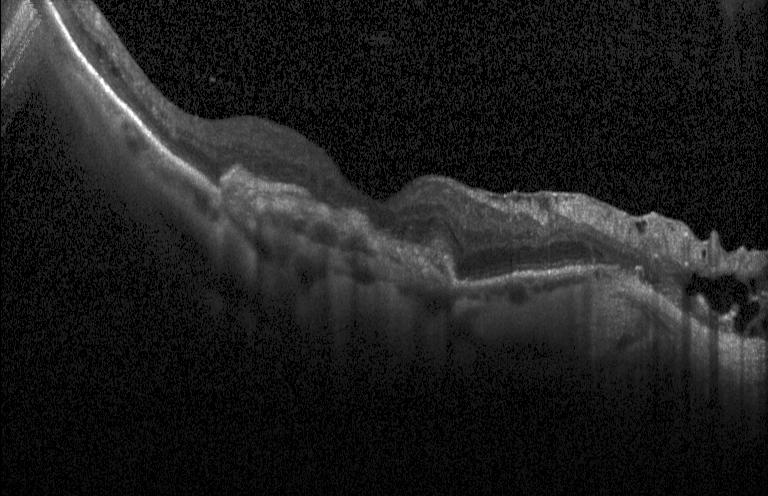 This B-scan demonstrates a choroidal neovascular membrane.